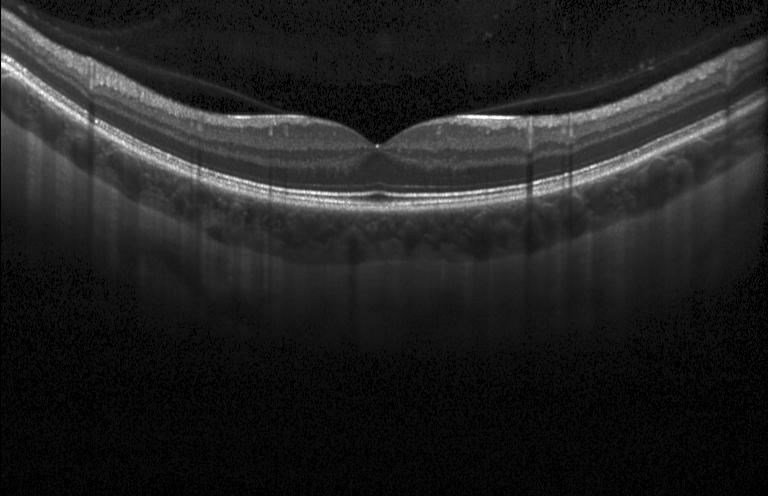 Retinal OCT B-scan, SD-OCT. Finding: no choroidal neovascularization, diabetic macular edema, or drusen.